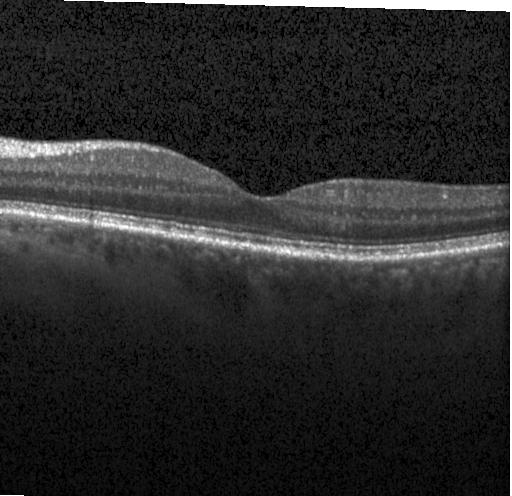
Retinal OCT B-scan · spectral-domain OCT · Heidelberg Spectralis OCT system — Impression: no evidence of CNV, DME, or drusen.